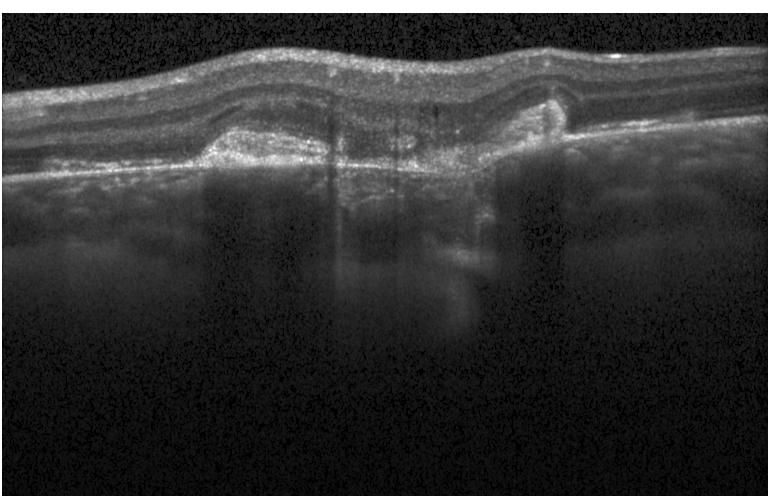

Spectral-domain OCT · retinal OCT B-scan. The scan shows a choroidal neovascular membrane.